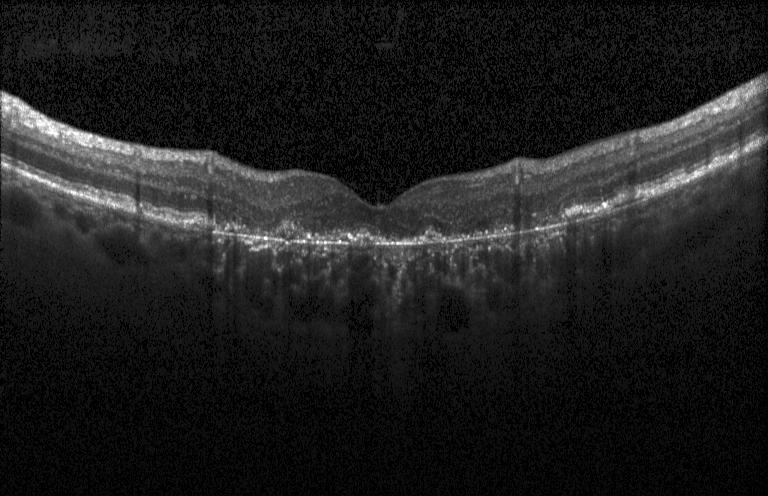 Spectral-domain optical coherence tomography, Heidelberg Spectralis, optical coherence tomography scan, fovea-centered
Diagnosis: choroidal neovascularization (CNV).